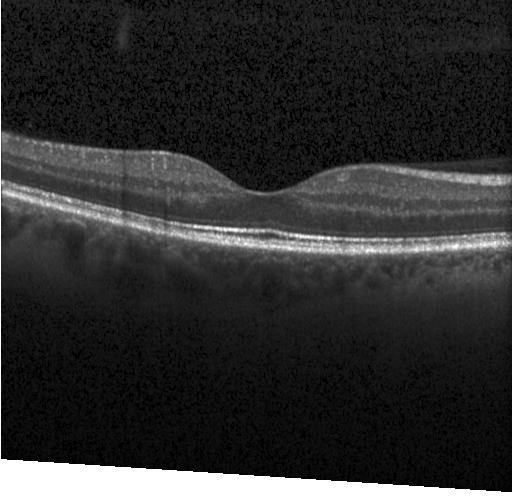
Macular scan, spectral-domain OCT, Heidelberg Spectralis, retinal OCT B-scan.
Dx: neither CNV, DME, nor drusen.